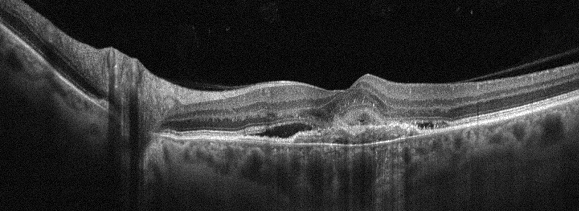 Oculus sinister. OCT B-scan. Macular scan.
Impression: AMD.